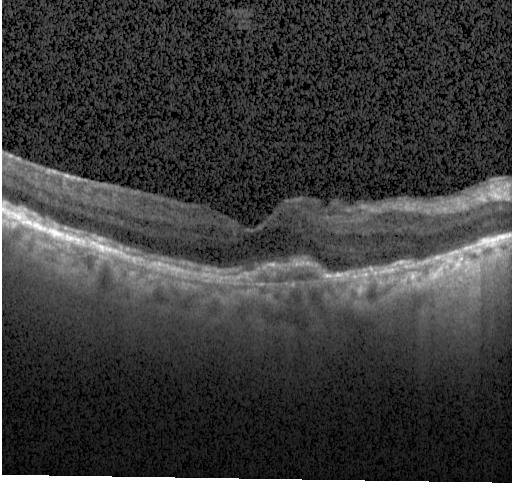 Centered on the fovea. Retinal OCT B-scan. Spectral-domain OCT. Acquired on a Heidelberg Spectralis.
Impression: a choroidal neovascular membrane.